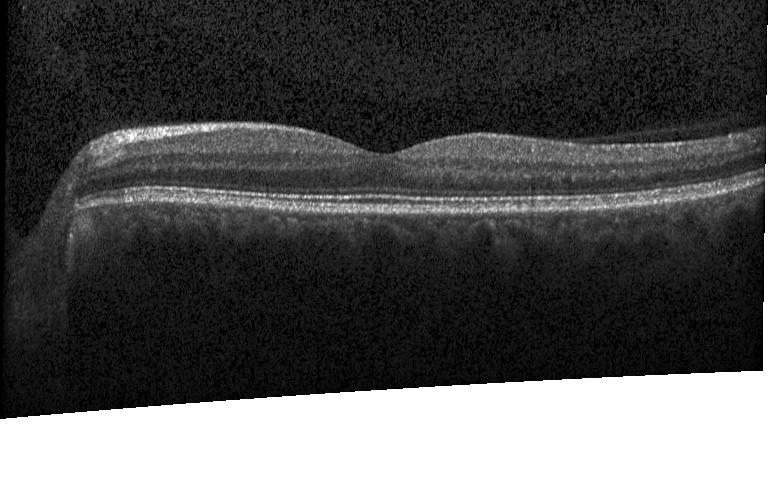
Retinal OCT cross-section, SD-OCT — Impression: neither CNV, DME, nor drusen.